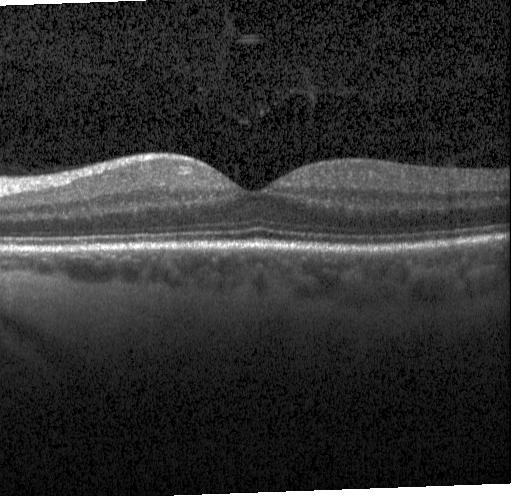
Spectral-domain OCT. Optical coherence tomography B-scan — Finding: neither CNV, DME, nor drusen.